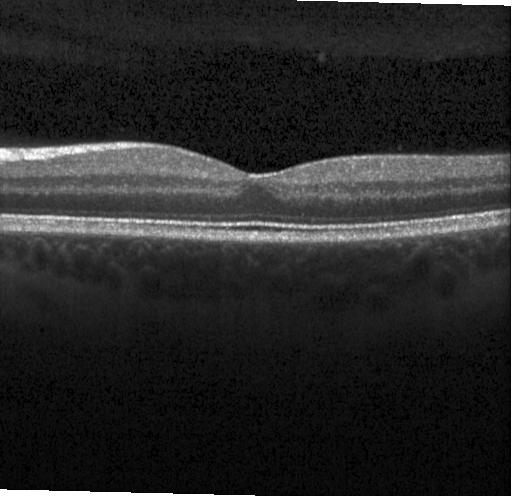

Spectral-domain OCT B-scan: no choroidal neovascularization, no diabetic macular edema, and no drusen.